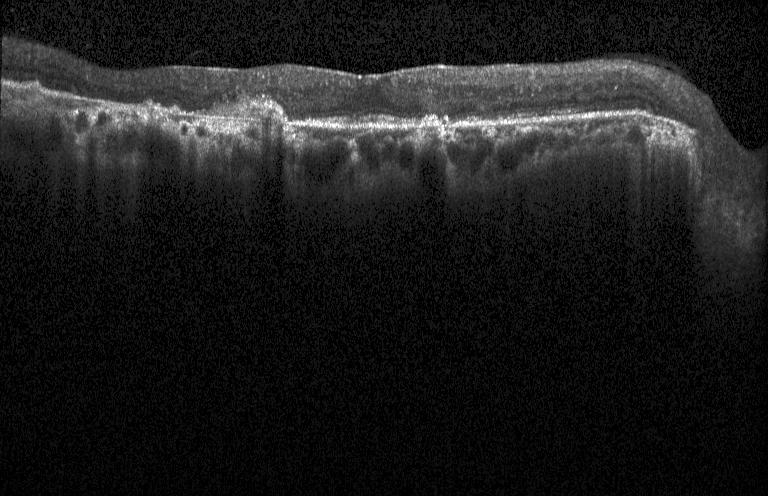

Retinal OCT cross-section. Impression: CNV.